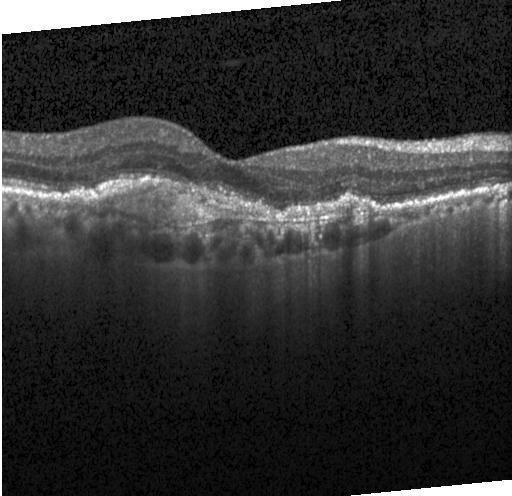

Instrument: Heidelberg Spectralis, spectral-domain OCT, optical coherence tomography scan, macular scan — Finding: a choroidal neovascular membrane.